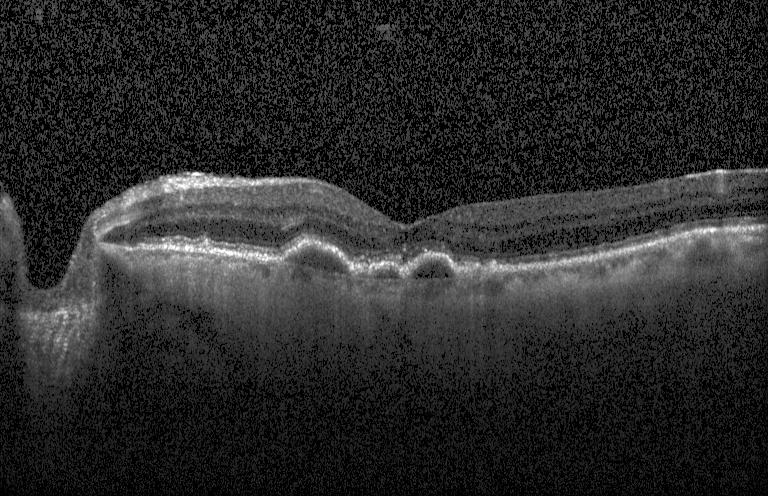

Retinal OCT cross-section · fovea-centered. Diagnosis: a choroidal neovascular membrane.